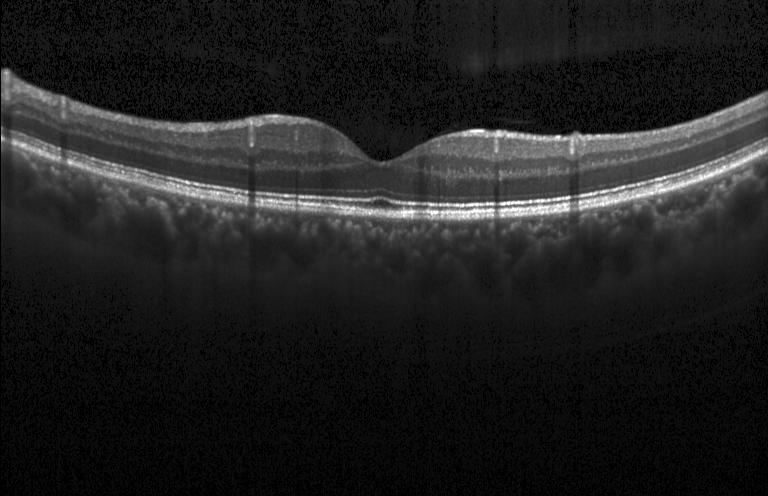
Optical coherence tomography B-scan; acquired on a Heidelberg Spectralis.
No choroidal neovascularization, no diabetic macular edema, and no drusen.